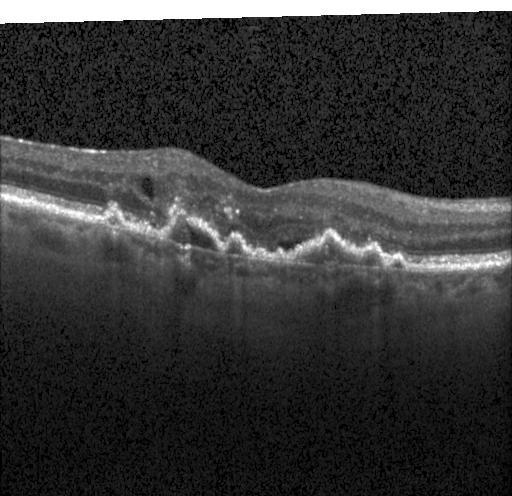

Assessment: a choroidal neovascular membrane.